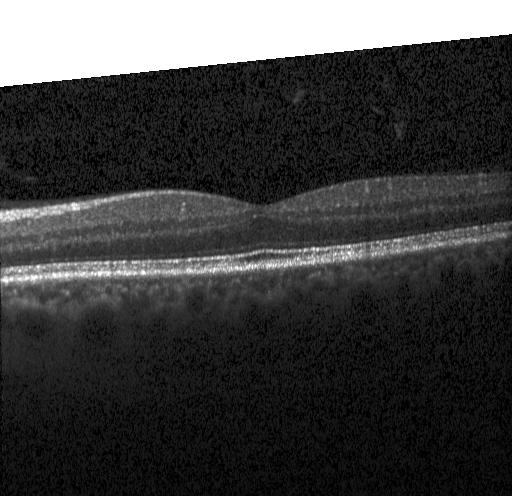
Optical coherence tomography scan.
Diagnosis: neither choroidal neovascularization, diabetic macular edema, nor drusen.